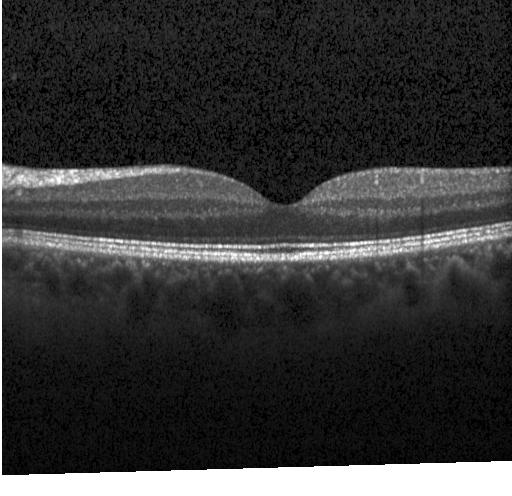

Fovea-centered; SD-OCT; optical coherence tomography B-scan — Diagnosis: no CNV, no DME, and no drusen.